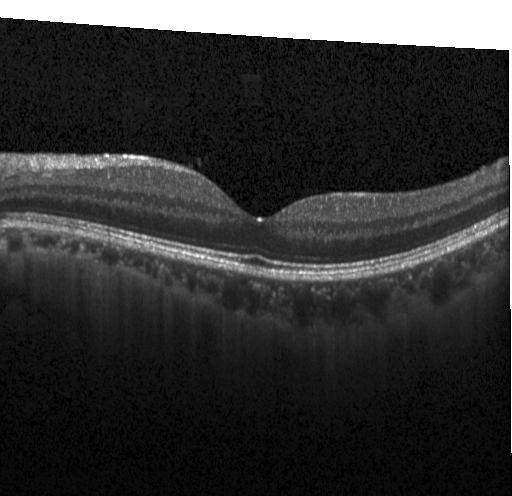
Macular OCT demonstrating no CNV, no DME, and no drusen.